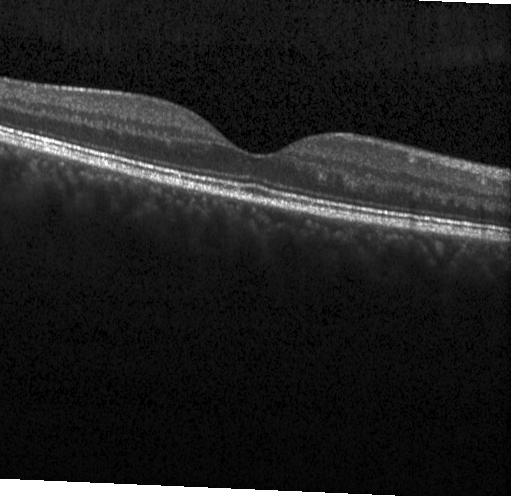 OCT line scan.
Finding: no evidence of choroidal neovascularization, diabetic macular edema, or drusen.